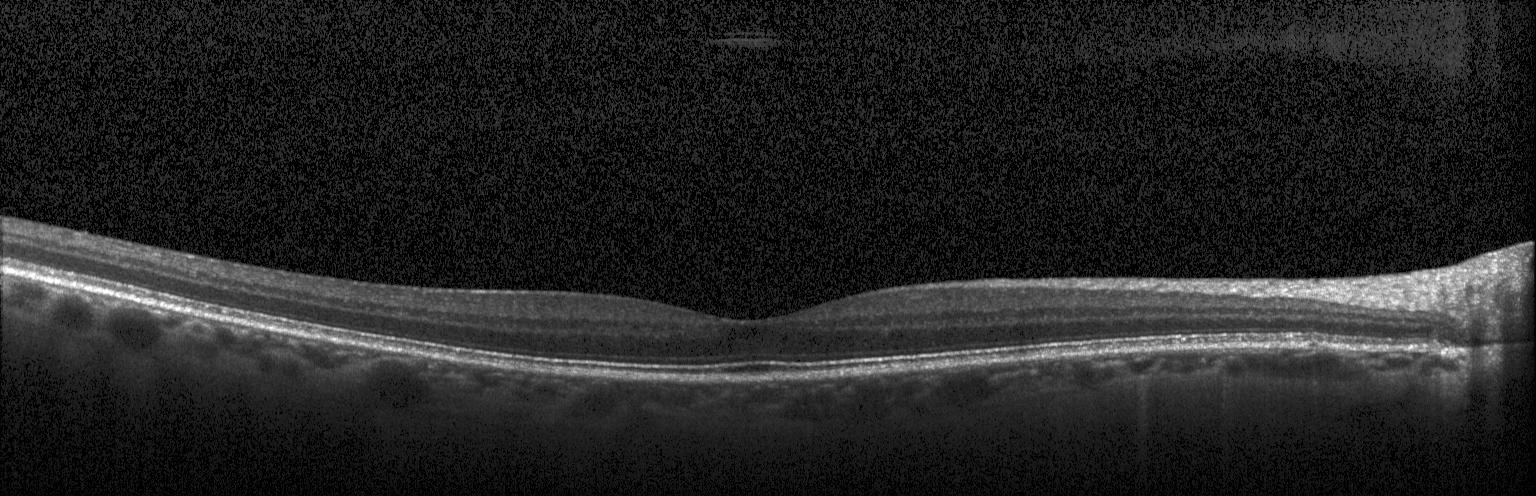

Spectral-domain OCT B-scan: neither CNV, DME, nor drusen.